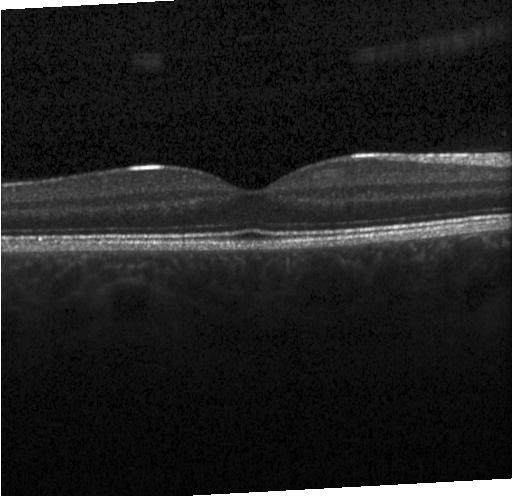

Macular OCT demonstrating neither choroidal neovascularization, diabetic macular edema, nor drusen.